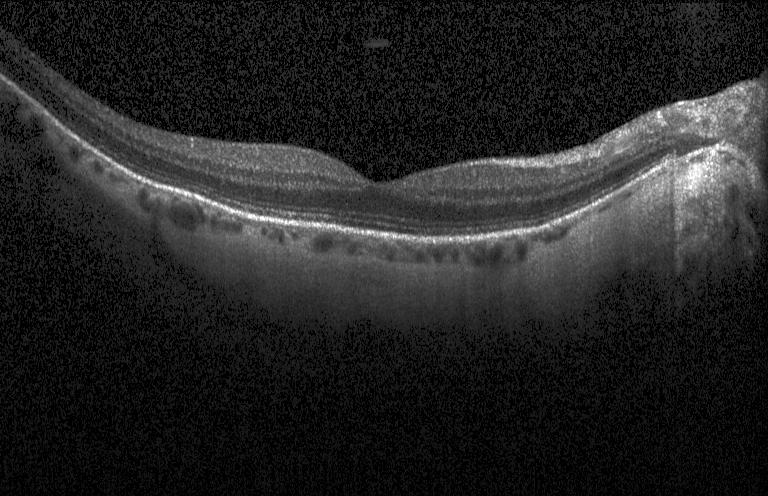 Retinal OCT cross-section showing no choroidal neovascularization, diabetic macular edema, or drusen.